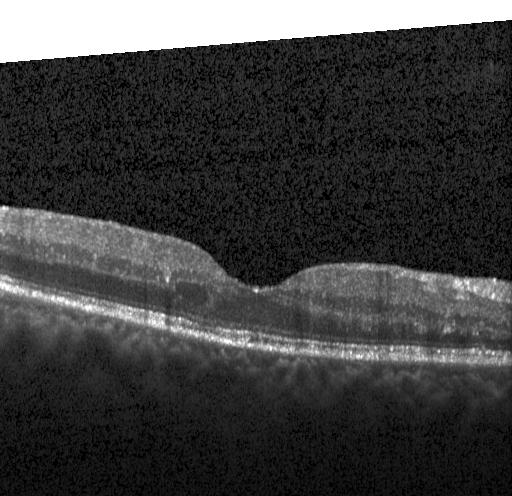

OCT finding: diabetic macular edema (DME).